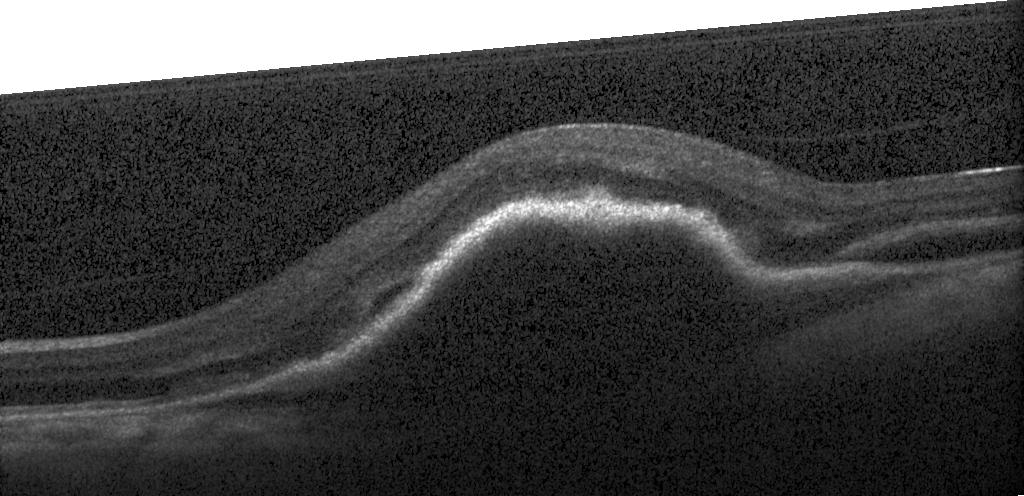 OCT B-scan showing choroidal neovascularization.